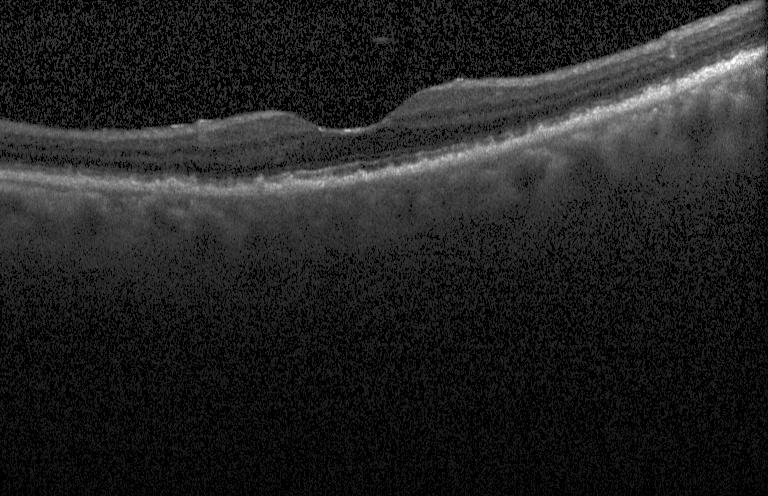

Centered on the fovea, acquired on a Heidelberg Spectralis, optical coherence tomography scan, spectral-domain OCT.
OCT finding: sub-RPE drusenoid deposits.